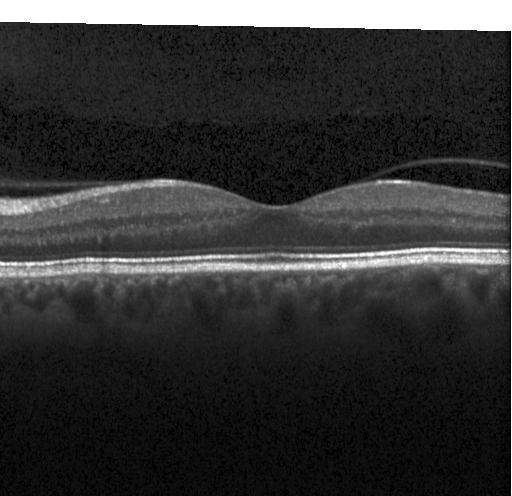 Spectral-domain OCT B-scan: no evidence of choroidal neovascularization, diabetic macular edema, or drusen.